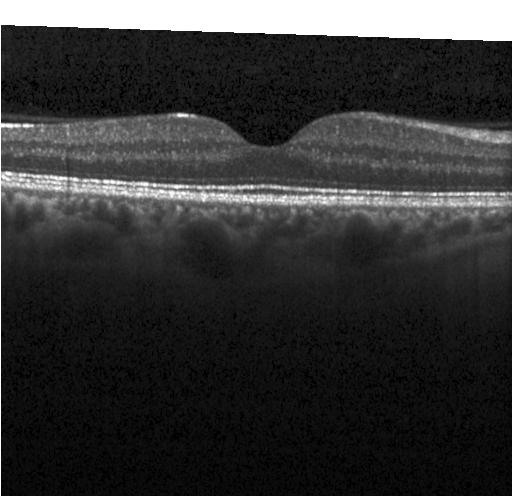
OCT B-scan showing no choroidal neovascularization, diabetic macular edema, or drusen.